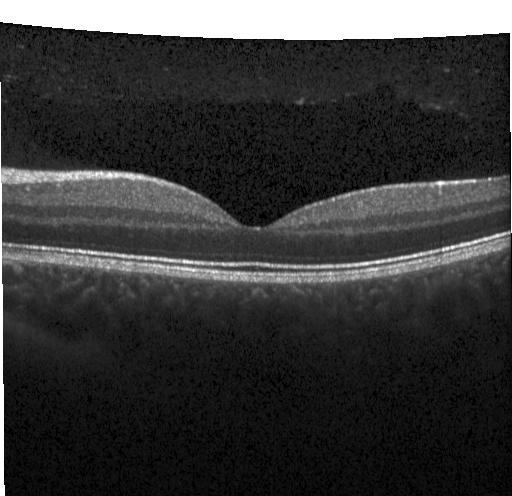
OCT B-scan. Macular OCT: no CNV, no DME, and no drusen.